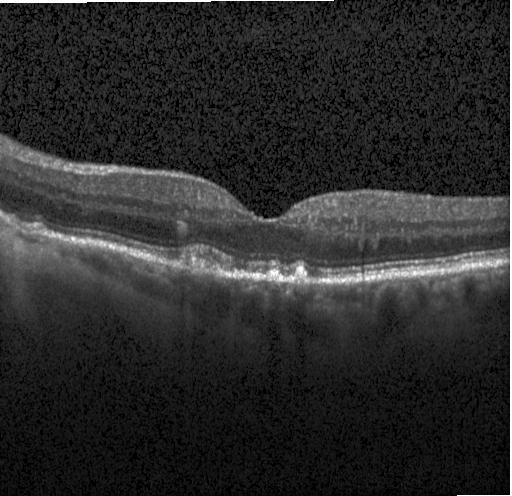

OCT B-scan · macular scan · acquired on a Heidelberg Spectralis
Dx: drusen.